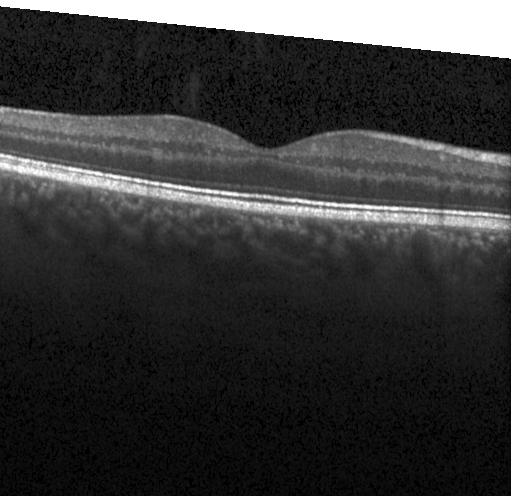 Impression: no choroidal neovascularization, diabetic macular edema, or drusen.